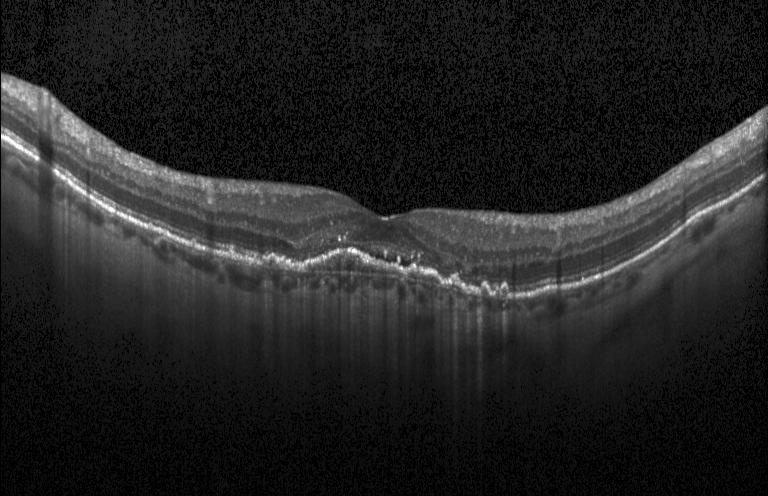

The scan shows a choroidal neovascular membrane.